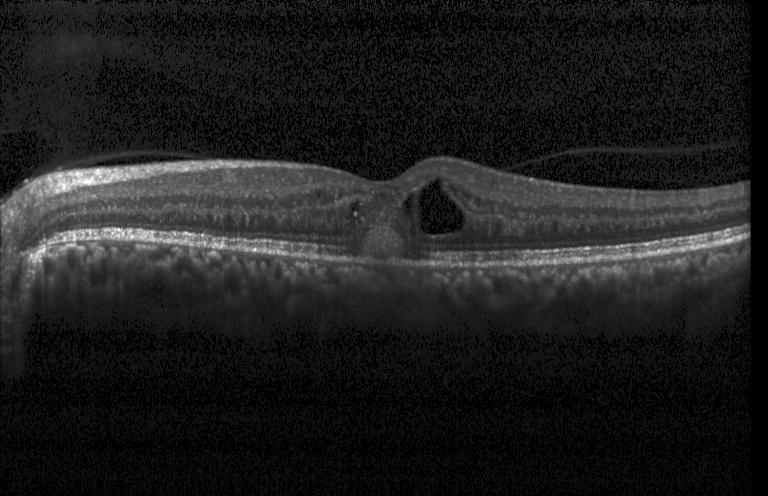 Instrument: Heidelberg Spectralis · fovea-centered · spectral-domain optical coherence tomography · OCT line scan.
Diagnosis: choroidal neovascularization.